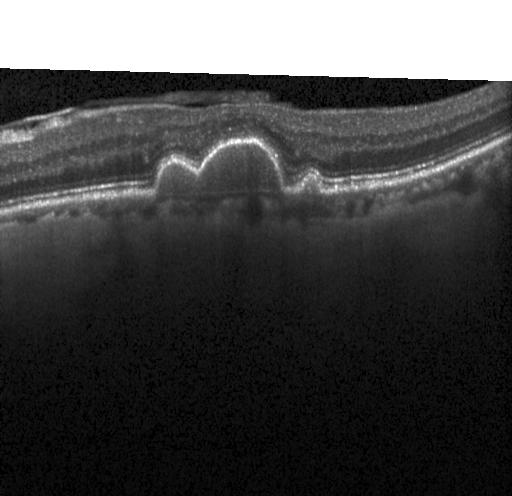

Fovea-centered. Retinal OCT cross-section.
Diagnosis: choroidal neovascularization (CNV).